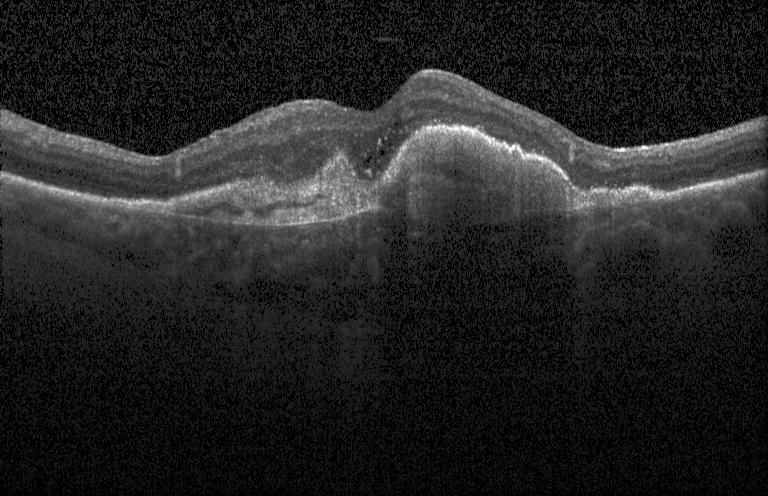
Instrument: Heidelberg Spectralis; horizontal scan through the fovea; OCT B-scan; SD-OCT
Diagnosis: a choroidal neovascular membrane.